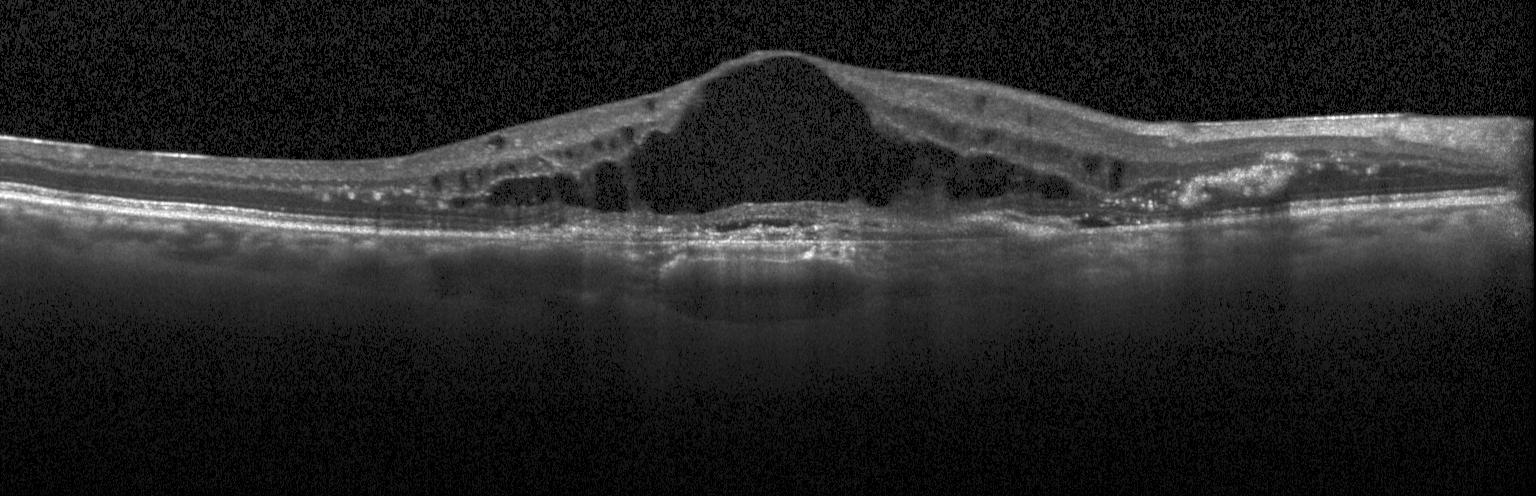
Heidelberg Spectralis. Retinal OCT B-scan — Diagnosis: CNV.